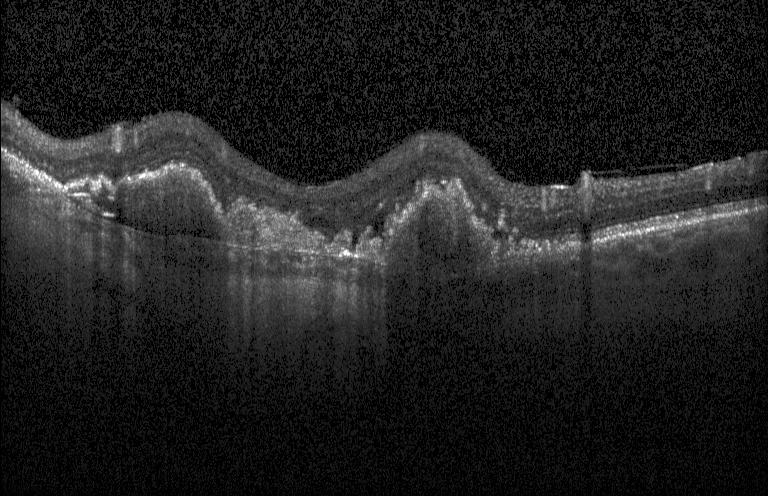
Optical coherence tomography scan.
Finding: a choroidal neovascular membrane.